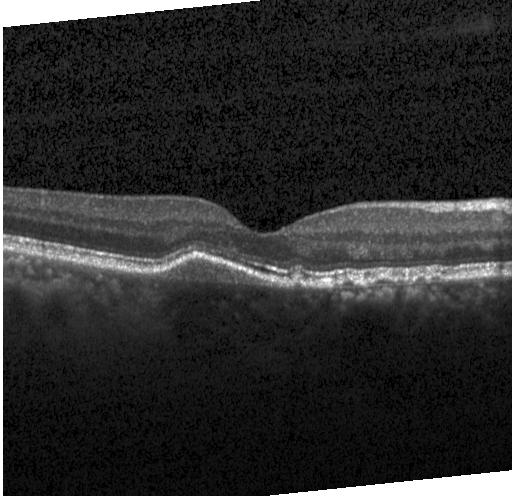

Assessment: drusen.